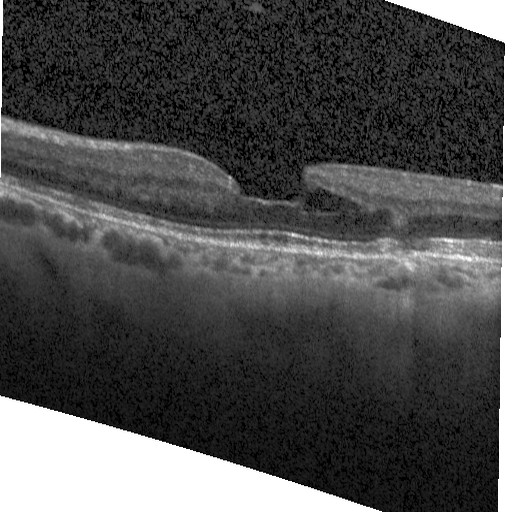
Macular scan, Heidelberg Spectralis, spectral-domain OCT, retinal OCT cross-section. Impression: diabetic macular edema.